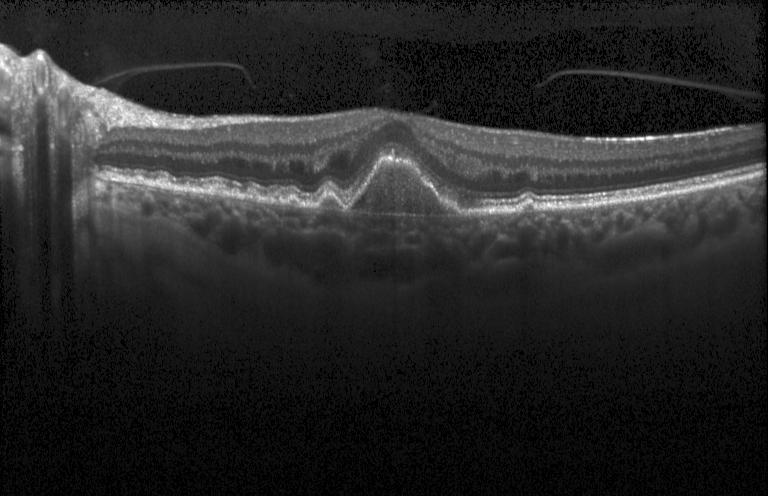 Optical coherence tomography B-scan, instrument: Heidelberg Spectralis — Macular OCT: CNV.